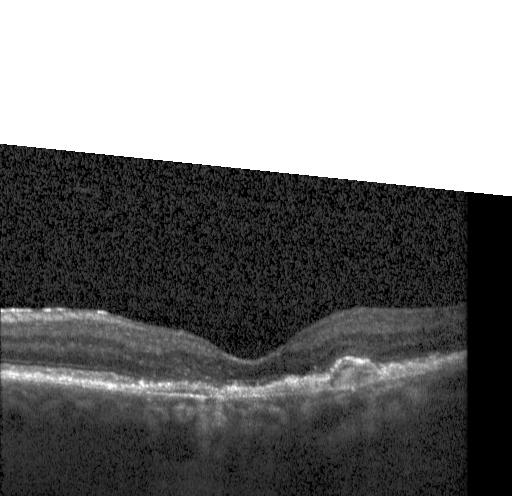

Spectral-domain OCT, retinal OCT B-scan, fovea-centered.
CNV.